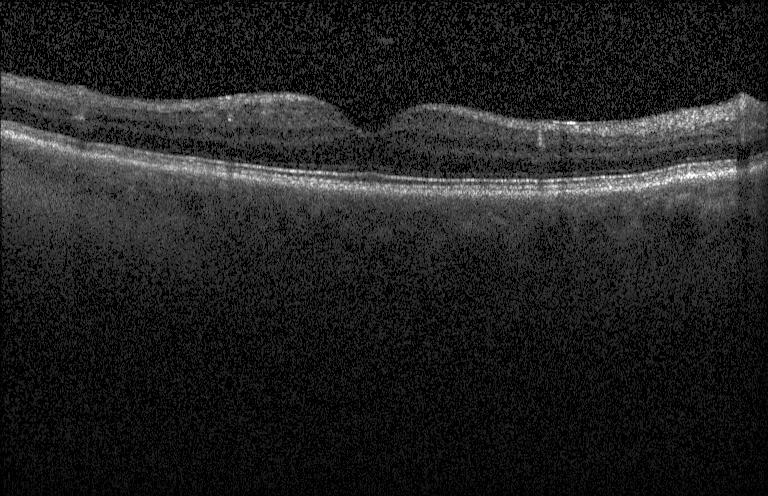

Retinal OCT cross-section showing no evidence of CNV, DME, or drusen.